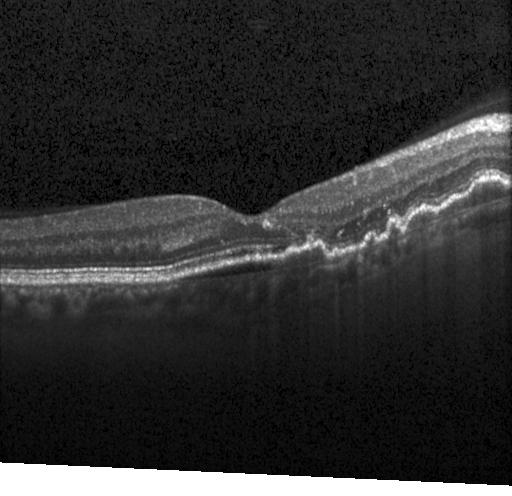
Optical coherence tomography B-scan, acquired on a Heidelberg Spectralis. A choroidal neovascular membrane.